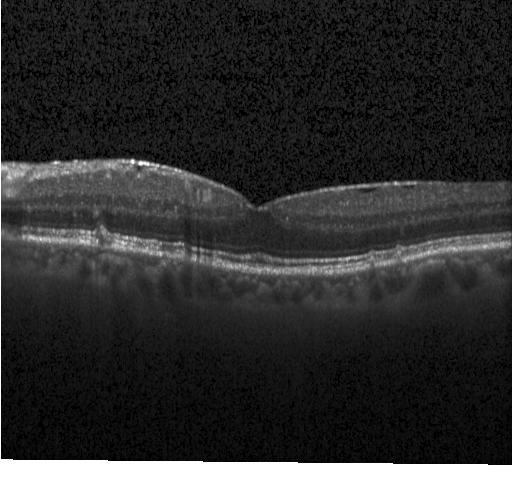 Finding: sub-RPE drusenoid deposits.